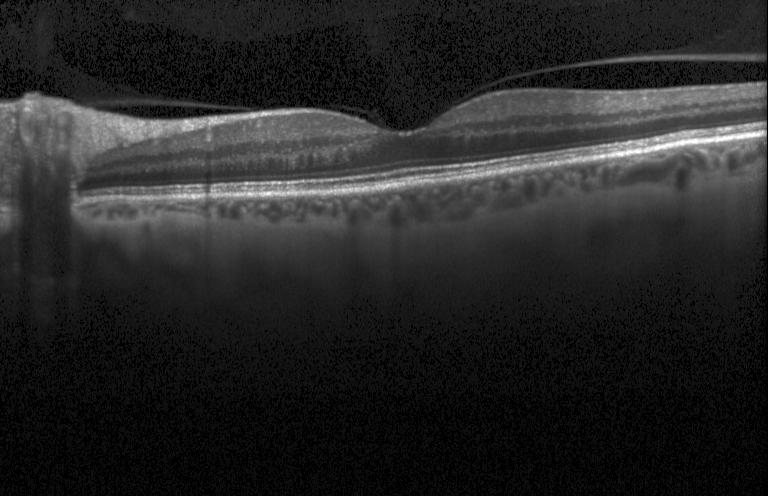

Spectral-domain optical coherence tomography, horizontal scan through the fovea, retinal OCT cross-section.
Impression: no choroidal neovascularization, no diabetic macular edema, and no drusen.